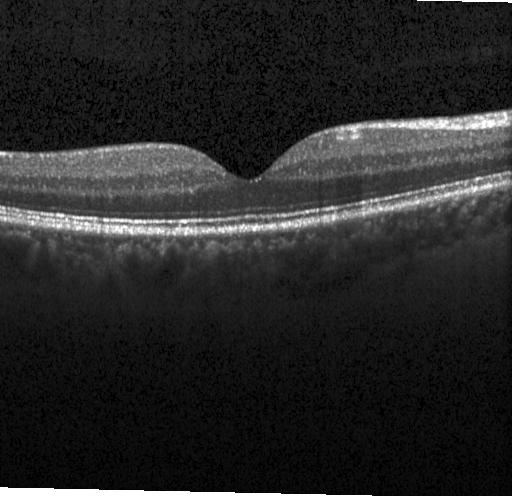
Dx: no choroidal neovascularization, diabetic macular edema, or drusen.